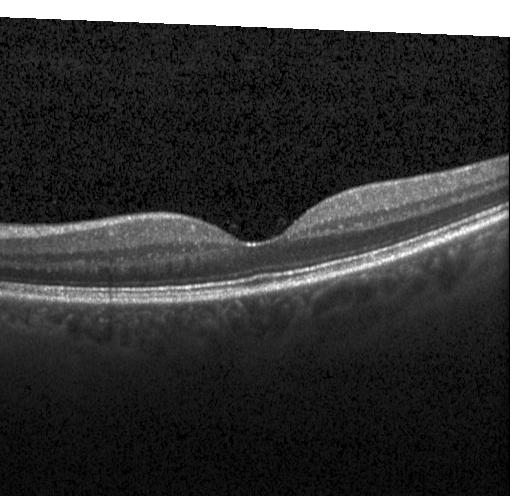

Diagnosis: no choroidal neovascularization, diabetic macular edema, or drusen.